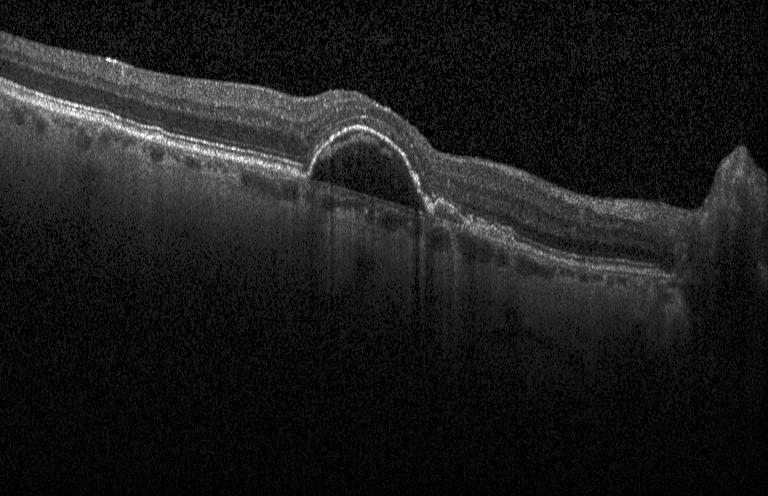 Diagnosis: CNV.